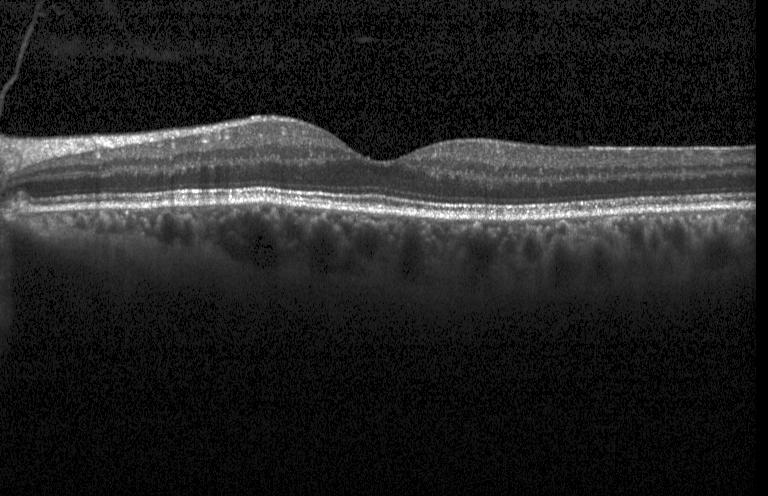
Impression: no choroidal neovascularization, no diabetic macular edema, and no drusen.